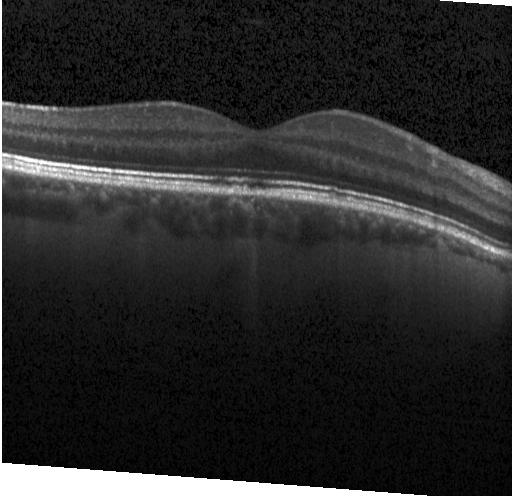
OCT line scan. Spectral-domain optical coherence tomography.
Diagnosis: no CNV, no DME, and no drusen.